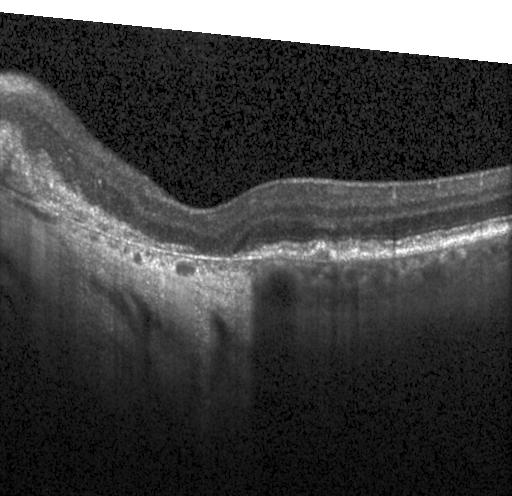 Fovea-centered. Retinal OCT B-scan — Impression: choroidal neovascularization (CNV).